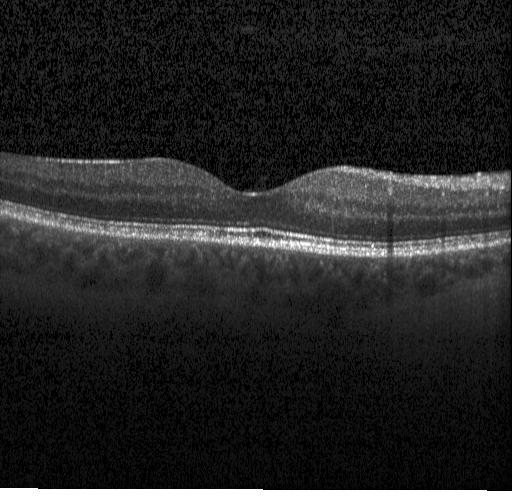
Instrument: Heidelberg Spectralis, macular scan, retinal OCT cross-section, spectral-domain OCT
Dx: neither choroidal neovascularization, diabetic macular edema, nor drusen.